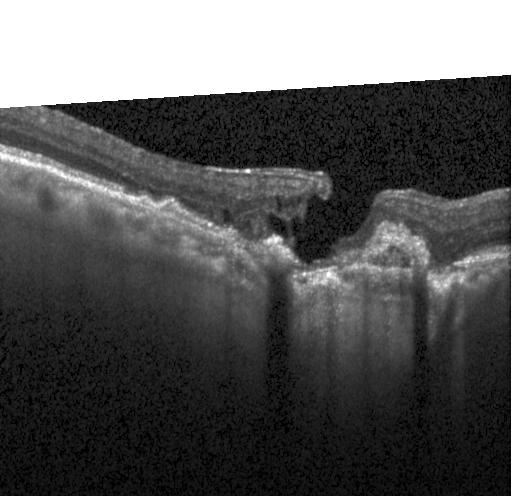 Retinal OCT cross-section showing choroidal neovascularization (CNV).